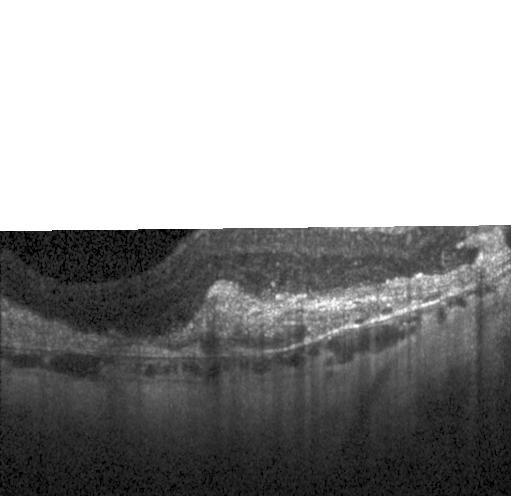 OCT B-scan · macular scan
Assessment: choroidal neovascularization (CNV).